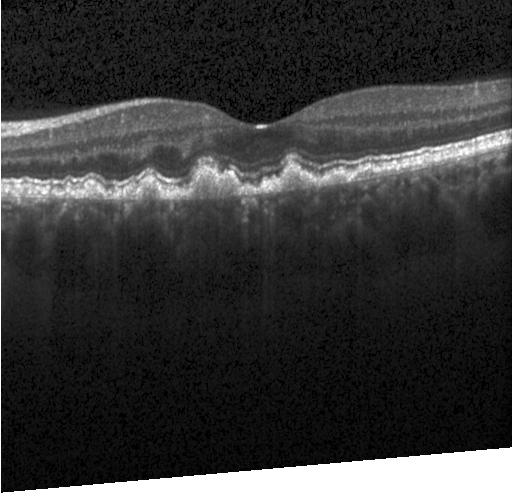
OCT B-scan showing drusen.